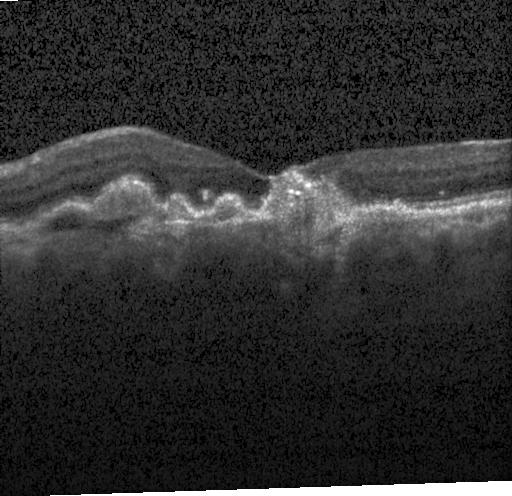

OCT B-scan
Impression: choroidal neovascularization (CNV).